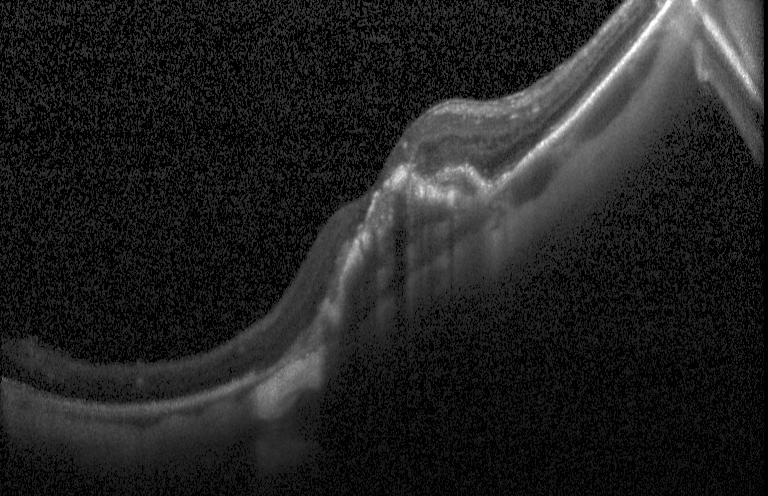

OCT line scan, macular scan.
This B-scan demonstrates a choroidal neovascular membrane.